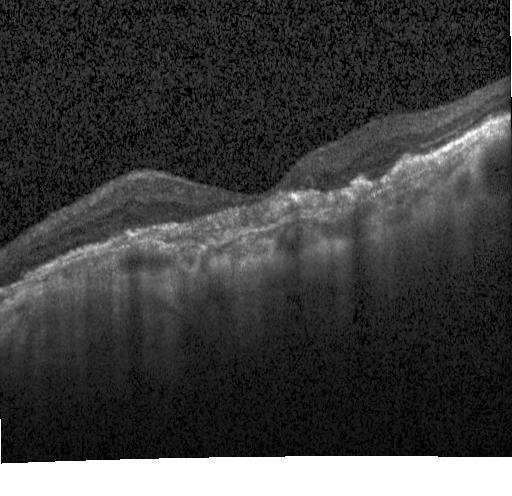 OCT B-scan showing choroidal neovascularization.